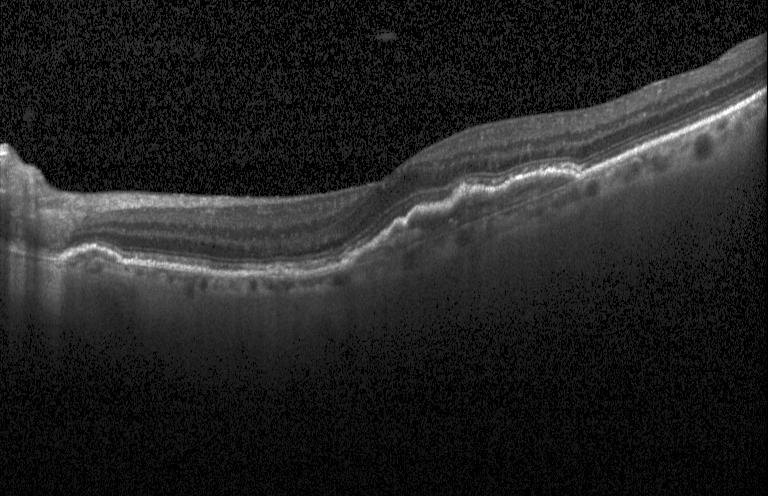

Dx: a choroidal neovascular membrane.